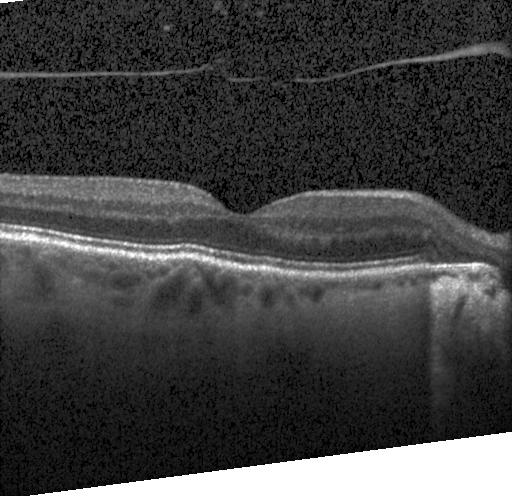

Spectral-domain OCT. Acquired on a Heidelberg Spectralis. Retinal OCT cross-section. Centered on the fovea — Impression: no evidence of choroidal neovascularization, diabetic macular edema, or drusen.